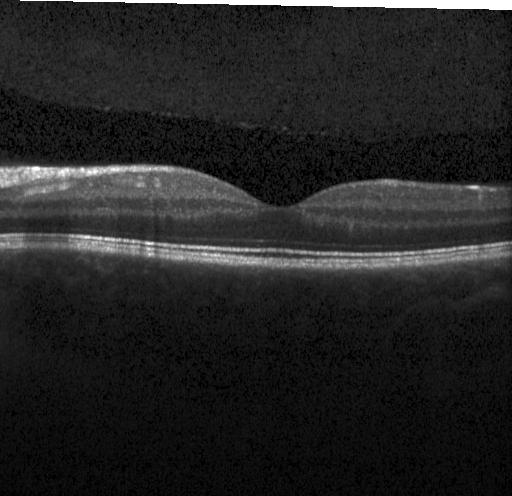

Finding: no evidence of choroidal neovascularization, diabetic macular edema, or drusen.